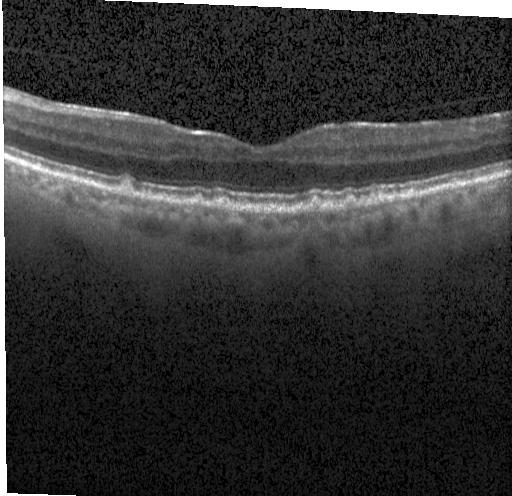 Diagnosis: drusen.